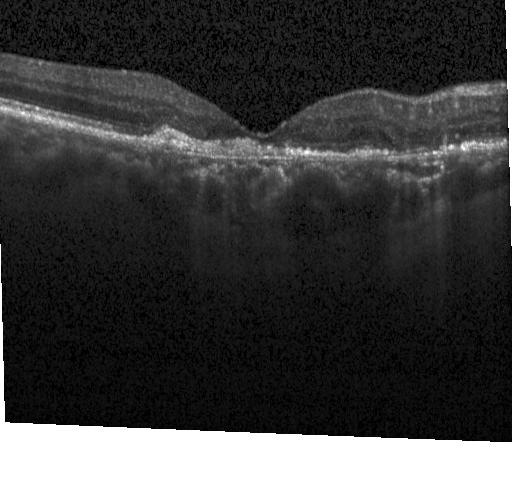
Finding: a choroidal neovascular membrane.